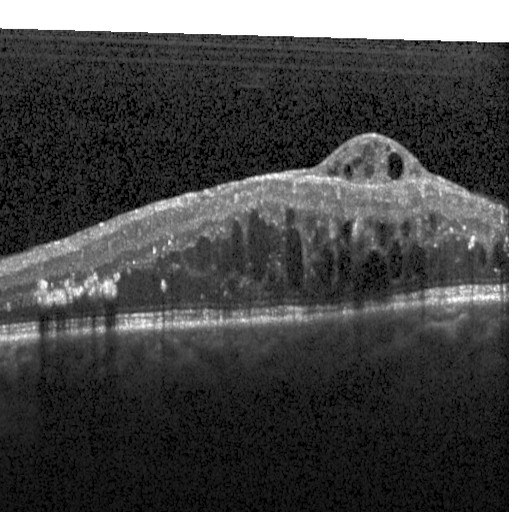 Optical coherence tomography scan; Heidelberg Spectralis OCT system.
Dx: diabetic macular edema.